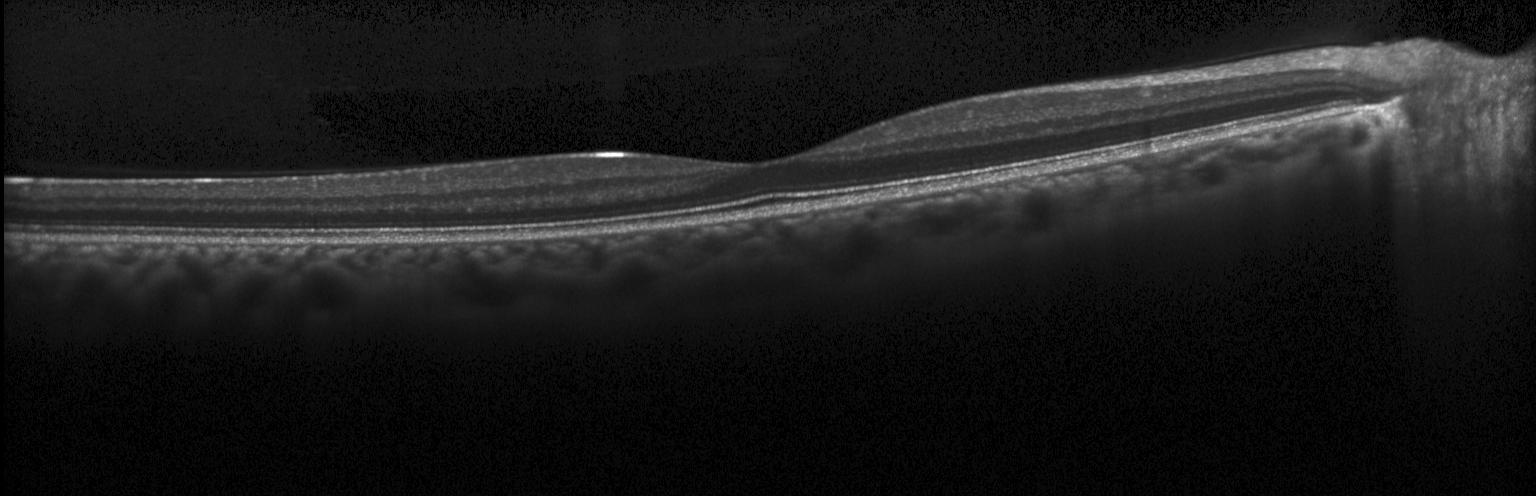 The scan shows no CNV, no DME, and no drusen.